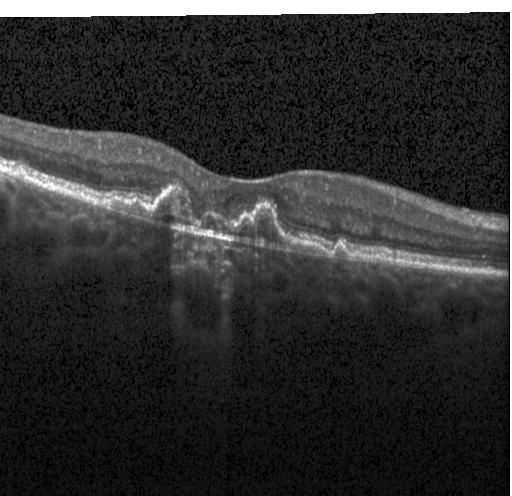

A choroidal neovascular membrane.